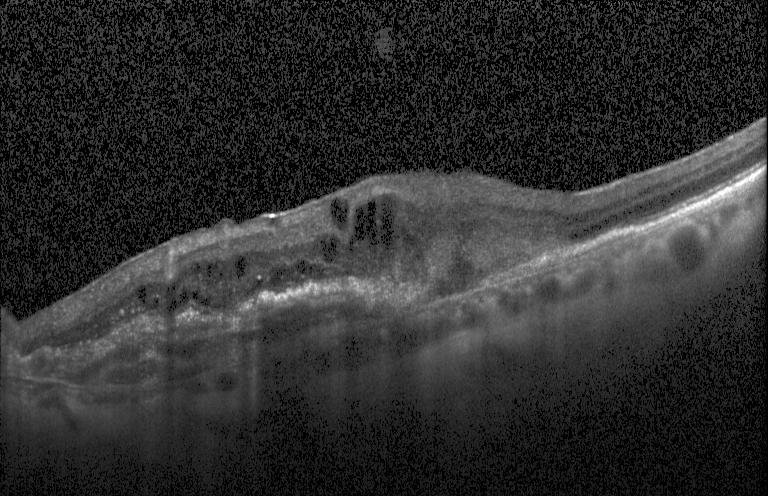

Instrument: Heidelberg Spectralis. Retinal OCT cross-section. Spectral-domain OCT. Through the macula. Diagnosis: choroidal neovascularization.